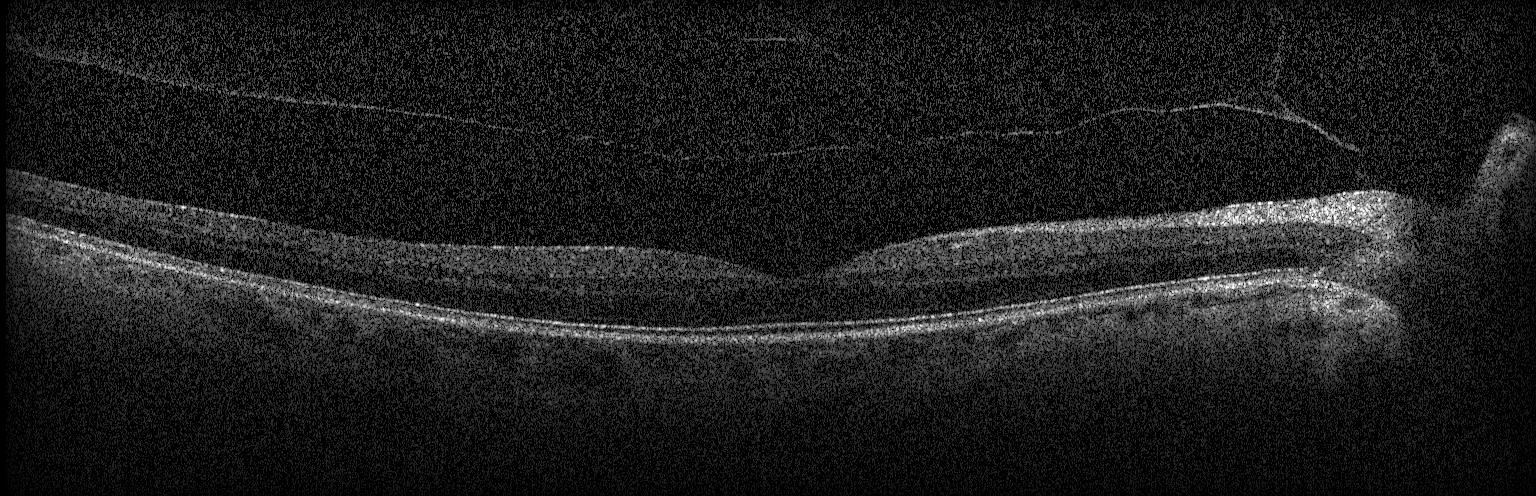
Spectral-domain OCT. Macular scan. Retinal OCT B-scan — Dx: neither choroidal neovascularization, diabetic macular edema, nor drusen.